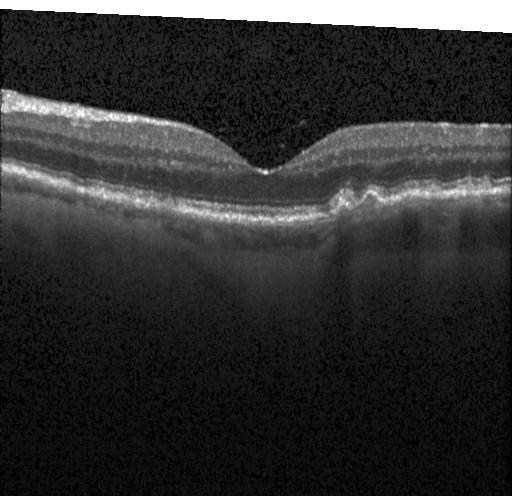
Retinal OCT B-scan
Impression: drusen.